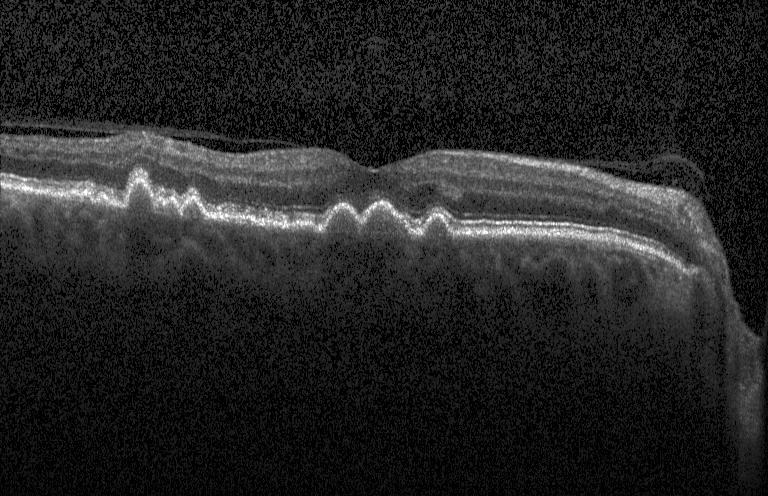
Spectral-domain OCT B-scan: multiple drusen.